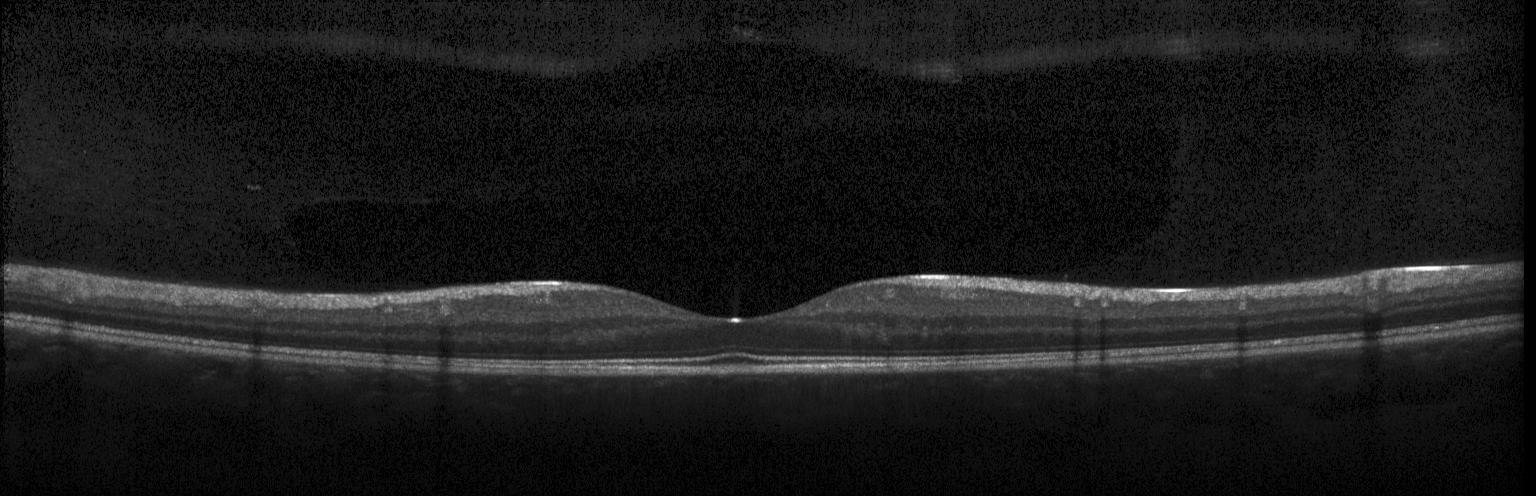

Heidelberg Spectralis, fovea-centered, OCT line scan, spectral-domain OCT — This B-scan demonstrates no CNV, no DME, and no drusen.